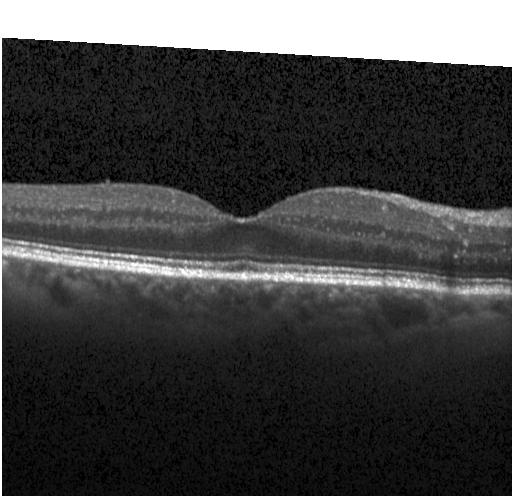

Spectral-domain OCT; centered on the fovea; optical coherence tomography scan. Impression: no evidence of CNV, DME, or drusen.